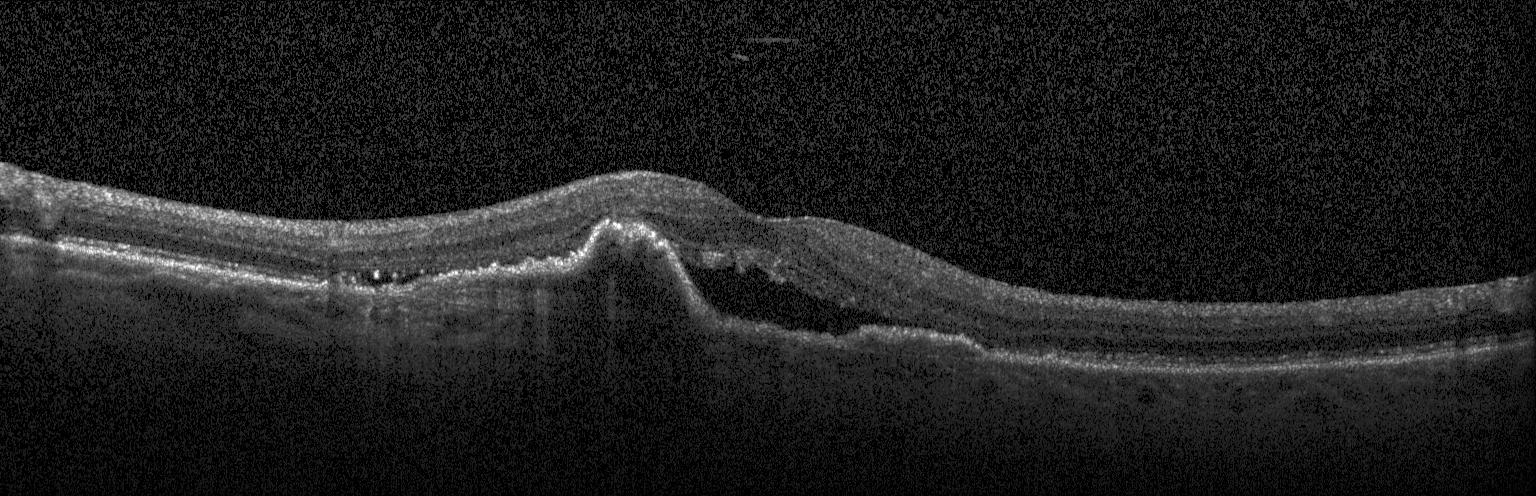 OCT B-scan; acquired on a Heidelberg Spectralis — Impression: choroidal neovascularization (CNV).